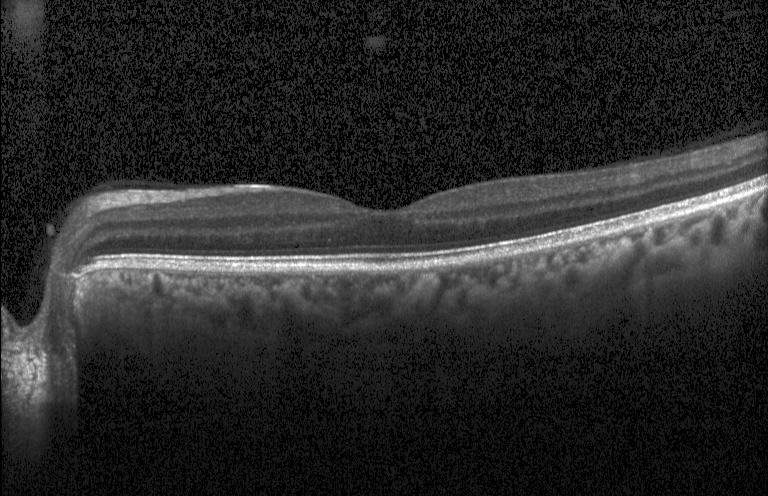 Instrument: Heidelberg Spectralis. Optical coherence tomography scan.
The scan shows neither CNV, DME, nor drusen.